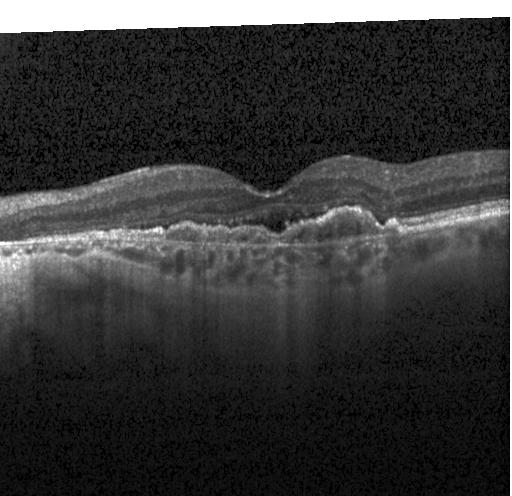
Retinal OCT cross-section showing CNV.